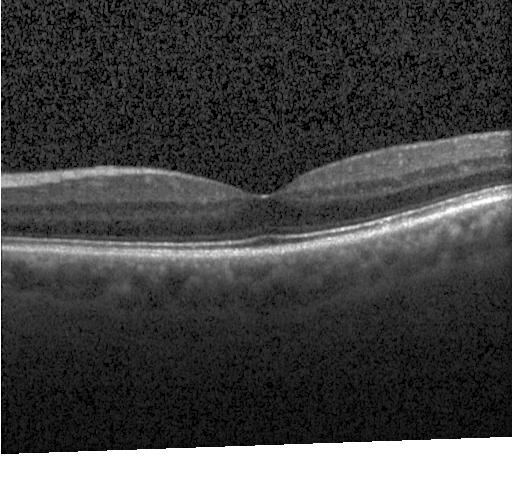 OCT finding: no evidence of choroidal neovascularization, diabetic macular edema, or drusen.